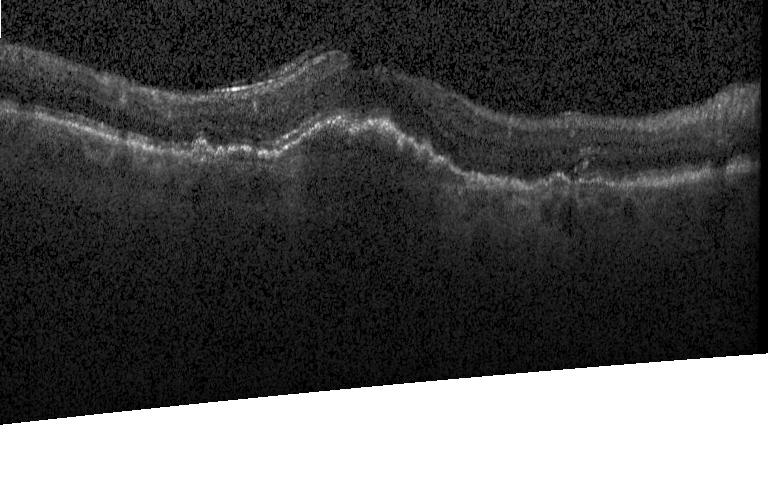
Optical coherence tomography B-scan, SD-OCT, fovea-centered, Heidelberg Spectralis OCT system — Dx: a choroidal neovascular membrane.